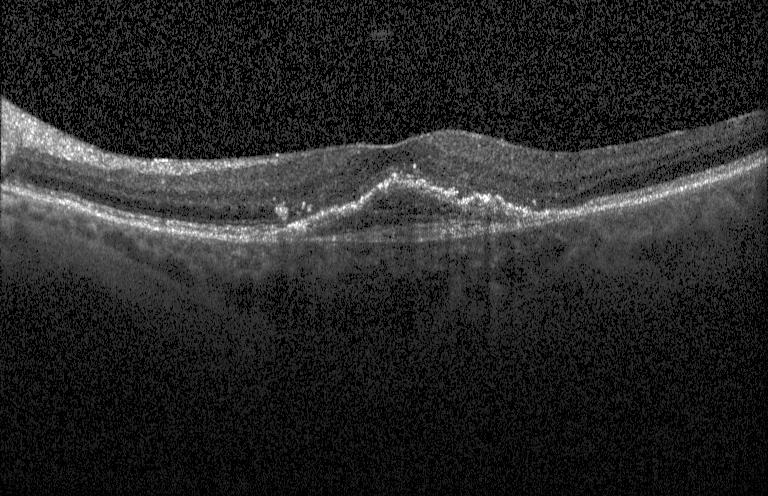 OCT B-scan. Heidelberg Spectralis OCT system
Dx: CNV.